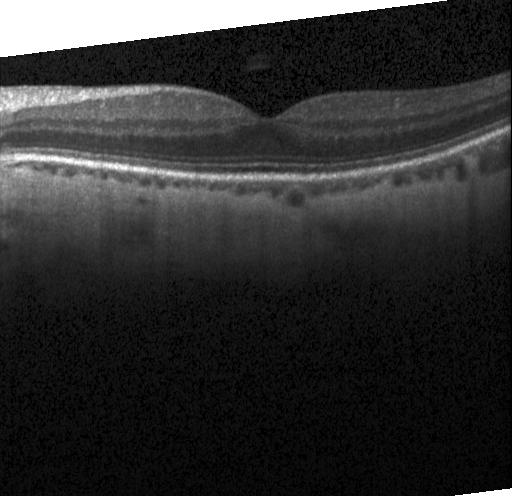
Macular OCT demonstrating no CNV, DME, or drusen.